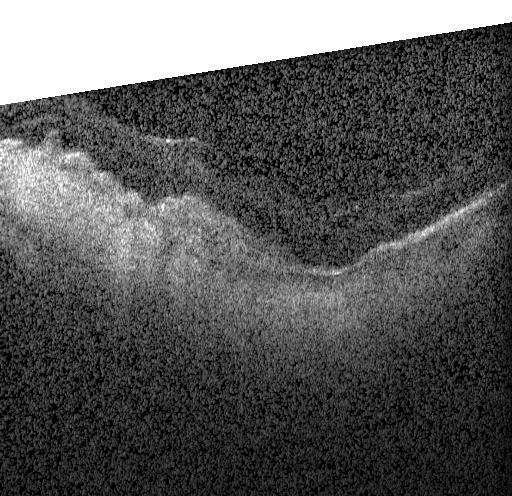

OCT B-scan.
Dx: a choroidal neovascular membrane.